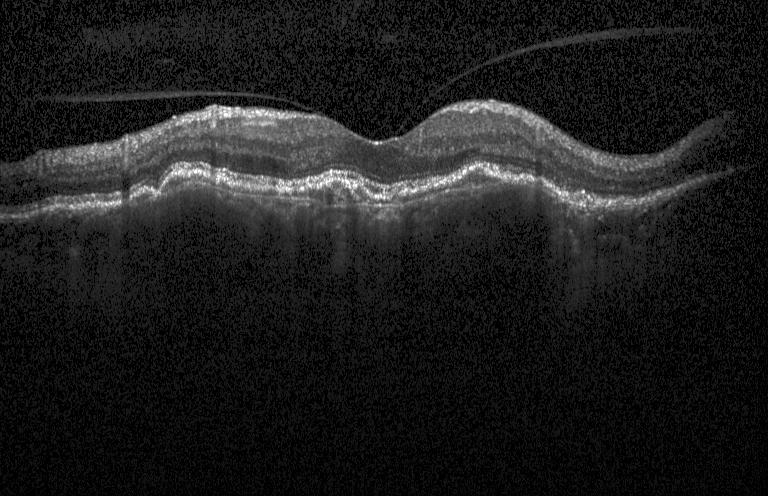 Spectral-domain optical coherence tomography; horizontal scan through the fovea; Heidelberg Spectralis OCT system; OCT B-scan.
The scan shows choroidal neovascularization (CNV).